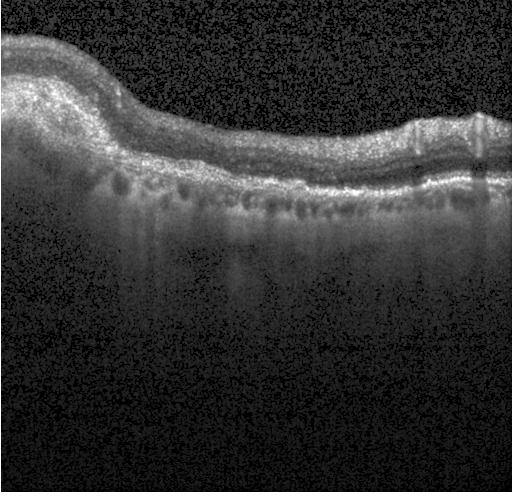 Optical coherence tomography B-scan
Finding: a choroidal neovascular membrane.